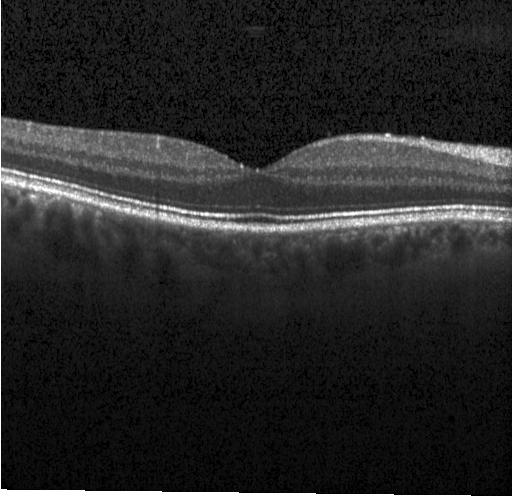
SD-OCT · optical coherence tomography scan · through the macula · Heidelberg Spectralis OCT system — Dx: no choroidal neovascularization, no diabetic macular edema, and no drusen.